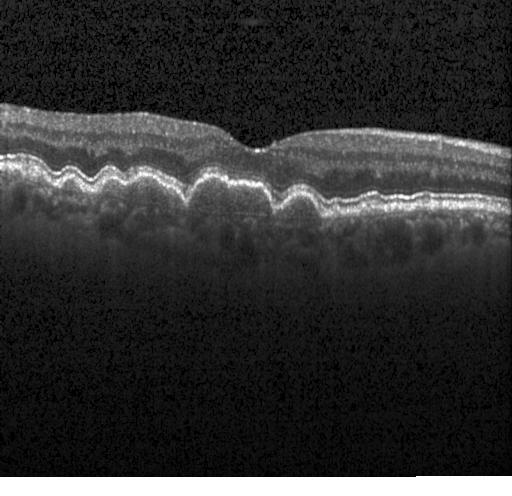

Heidelberg Spectralis; OCT line scan; SD-OCT; macular scan
Finding: multiple drusen.